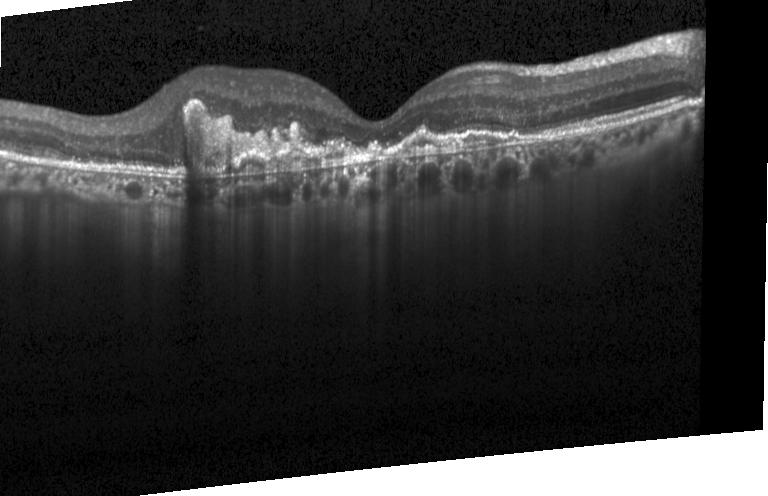
Finding: a choroidal neovascular membrane.